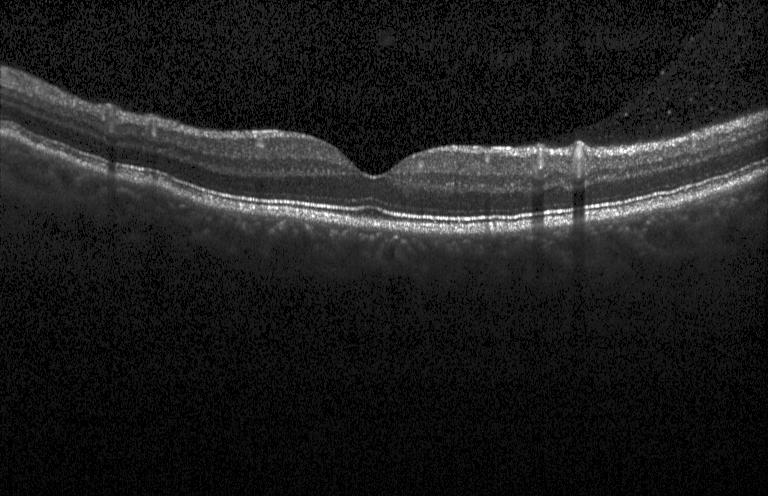 Heidelberg Spectralis. SD-OCT. OCT line scan — Diagnosis: neither choroidal neovascularization, diabetic macular edema, nor drusen.